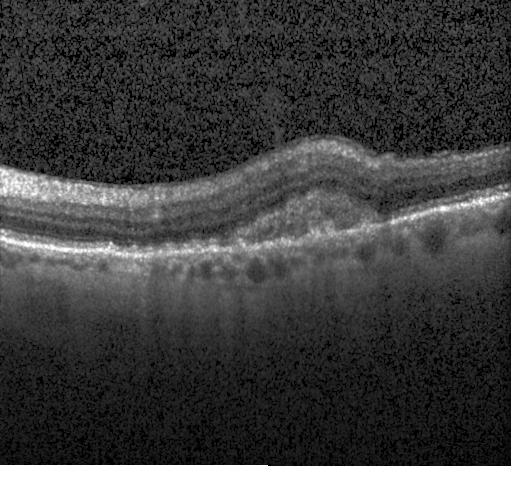 Impression: a choroidal neovascular membrane.